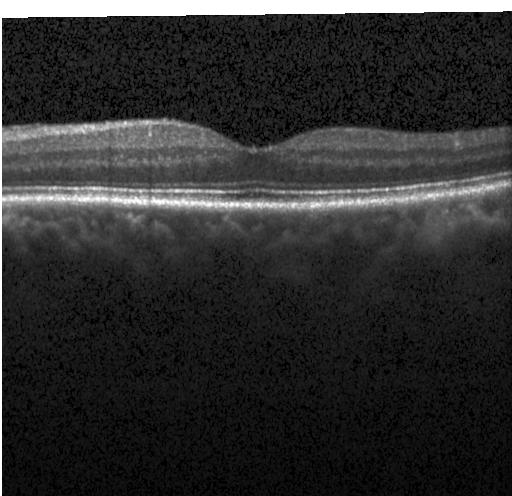

Finding: no evidence of choroidal neovascularization, diabetic macular edema, or drusen.